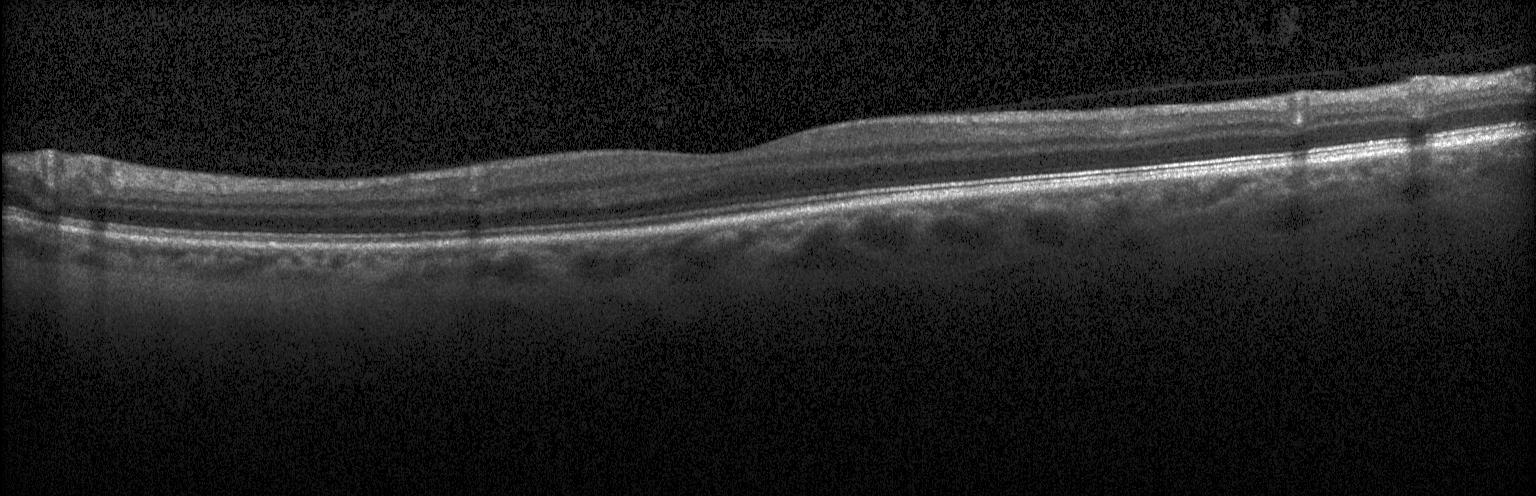
Finding: no CNV, no DME, and no drusen.